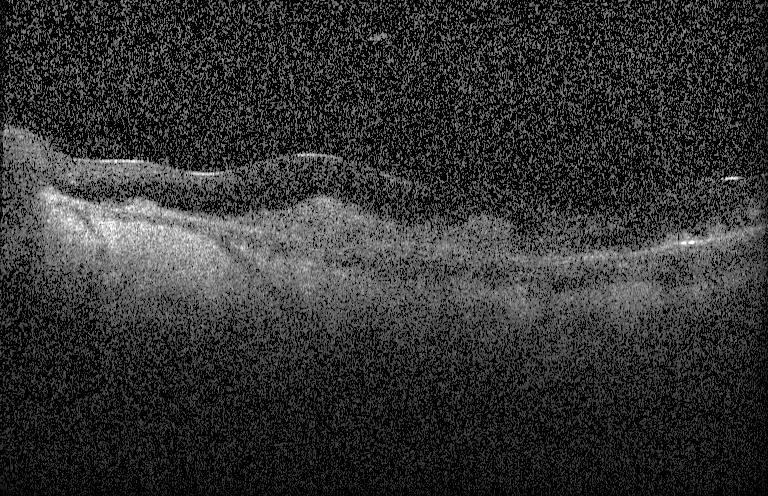

Optical coherence tomography B-scan; horizontal scan through the fovea; instrument: Heidelberg Spectralis
Impression: choroidal neovascularization.